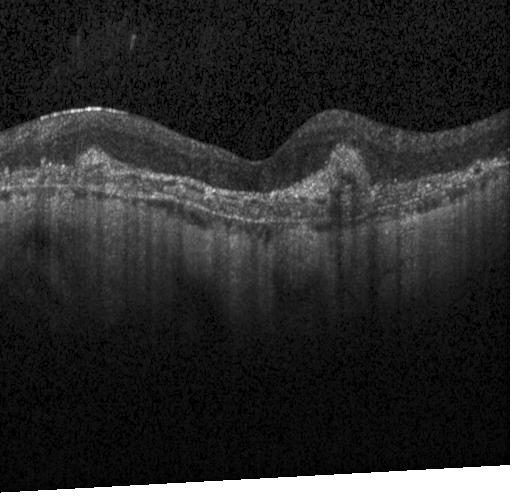 Through the macula. Retinal OCT cross-section. Instrument: Heidelberg Spectralis
Finding: choroidal neovascularization.